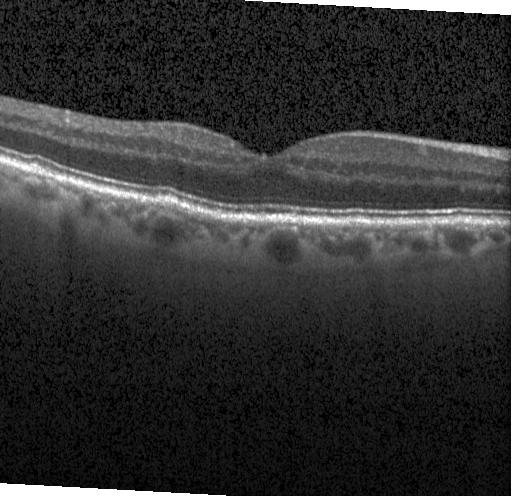 SD-OCT, optical coherence tomography scan. Finding: sub-RPE drusenoid deposits.